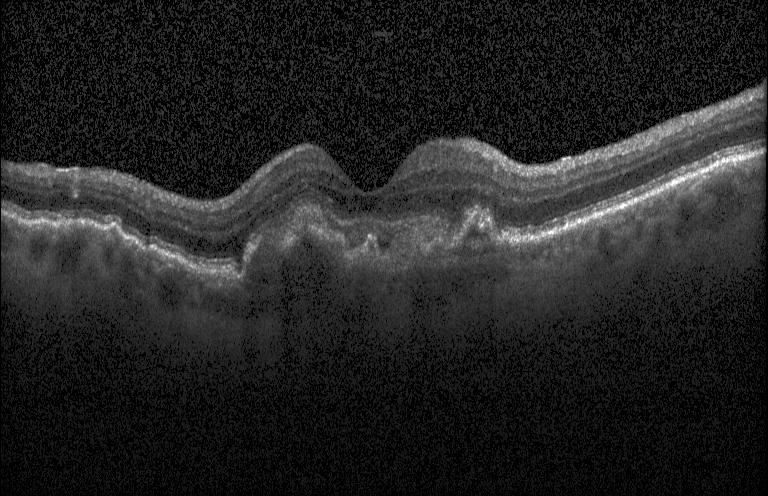 Heidelberg Spectralis. OCT B-scan. Finding: choroidal neovascularization.